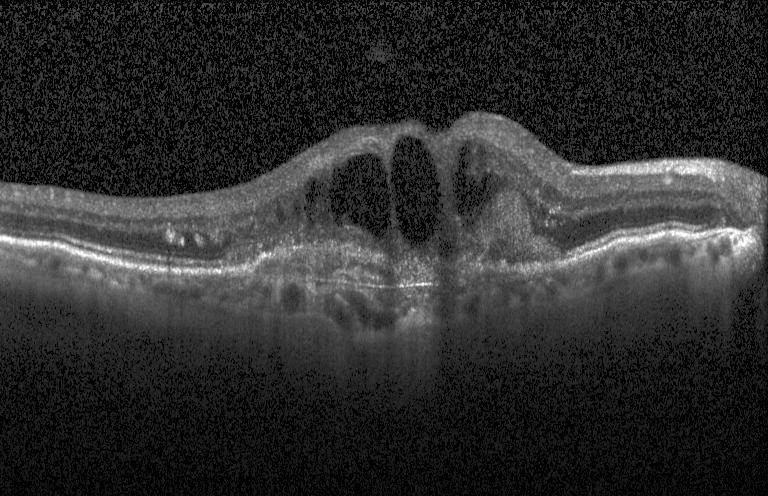
Macular scan; optical coherence tomography B-scan; SD-OCT — Dx: CNV.